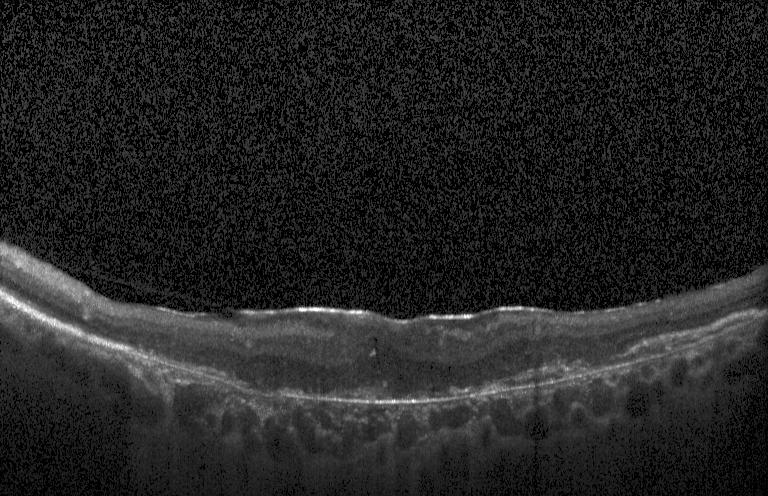
OCT B-scan · spectral-domain OCT — Impression: a choroidal neovascular membrane.